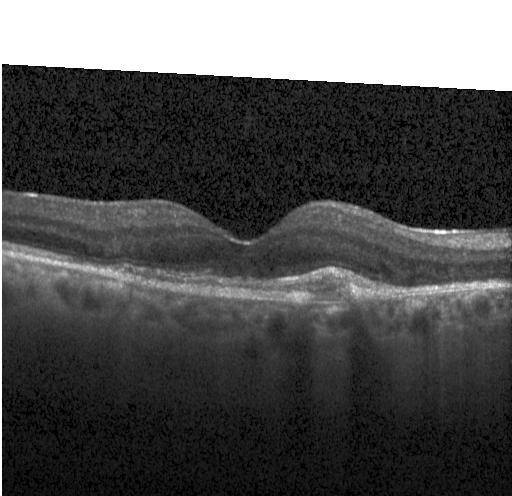
OCT B-scan
Finding: CNV.